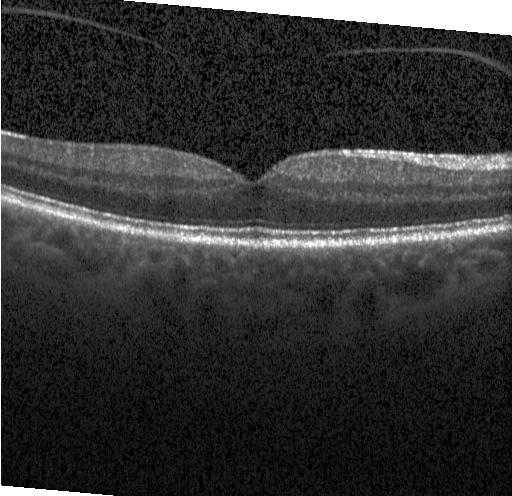

Acquired on a Heidelberg Spectralis; retinal OCT B-scan; horizontal scan through the fovea. Dx: no CNV, no DME, and no drusen.